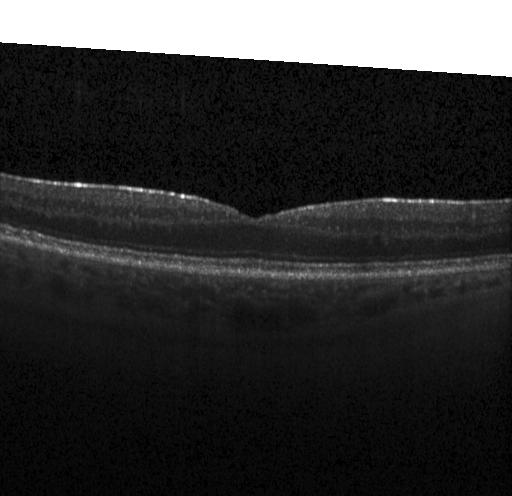
Centered on the fovea, Heidelberg Spectralis, spectral-domain OCT, OCT line scan — No choroidal neovascularization, no diabetic macular edema, and no drusen.